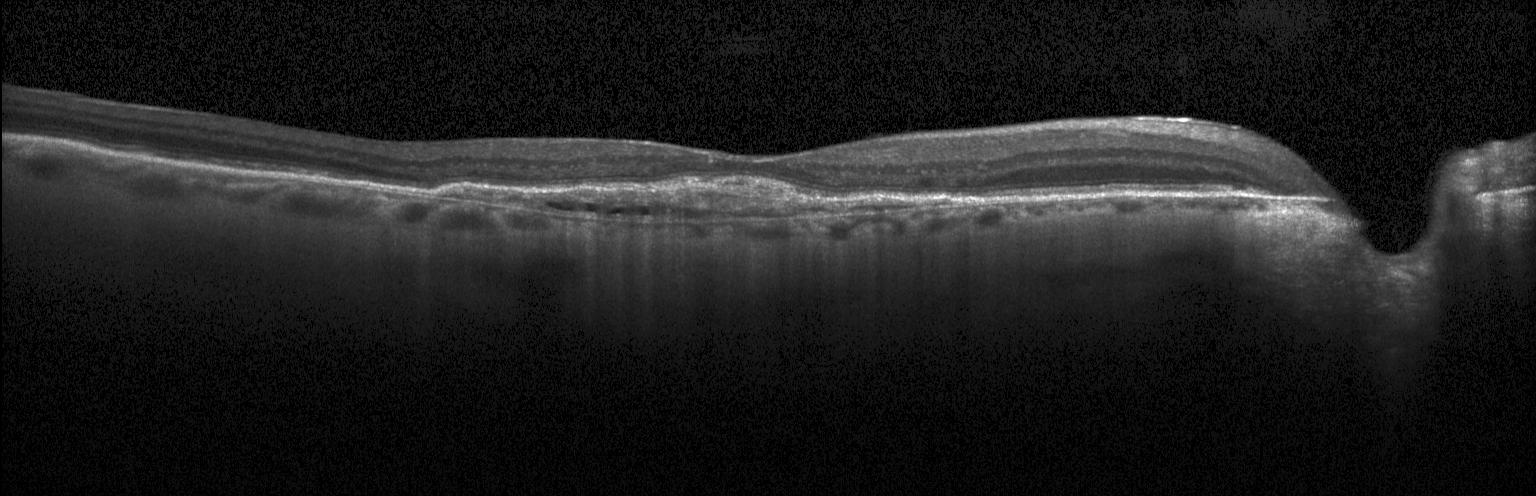

This B-scan demonstrates choroidal neovascularization.